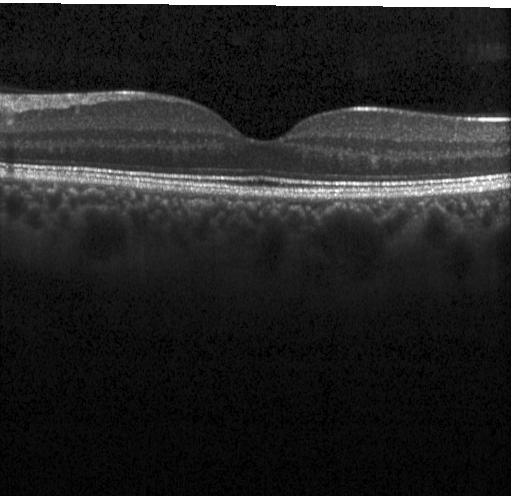 Retinal OCT B-scan, centered on the fovea, spectral-domain optical coherence tomography, Heidelberg Spectralis
Assessment: no evidence of choroidal neovascularization, diabetic macular edema, or drusen.